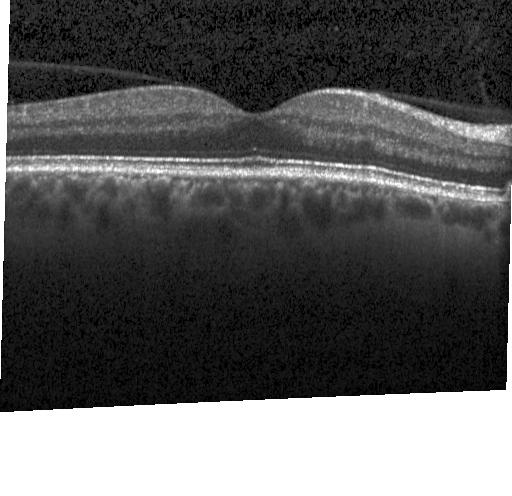
Finding: no evidence of choroidal neovascularization, diabetic macular edema, or drusen.